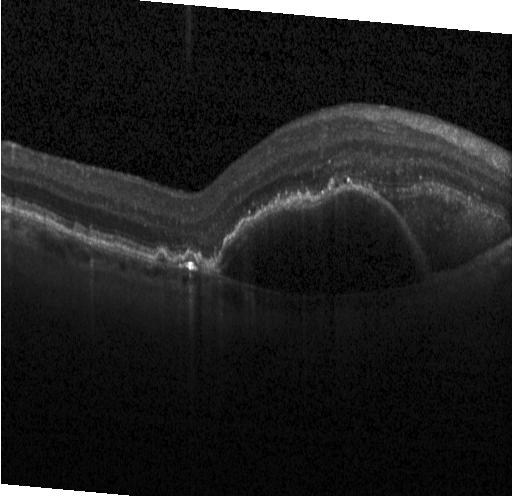
OCT B-scan showing choroidal neovascularization.